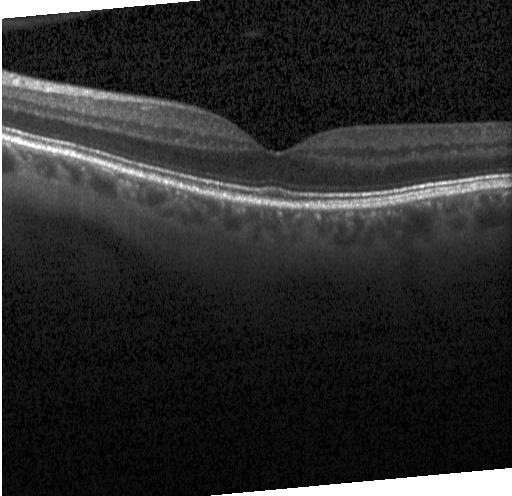

Optical coherence tomography B-scan. Instrument: Heidelberg Spectralis — Macular OCT: no CNV, no DME, and no drusen.